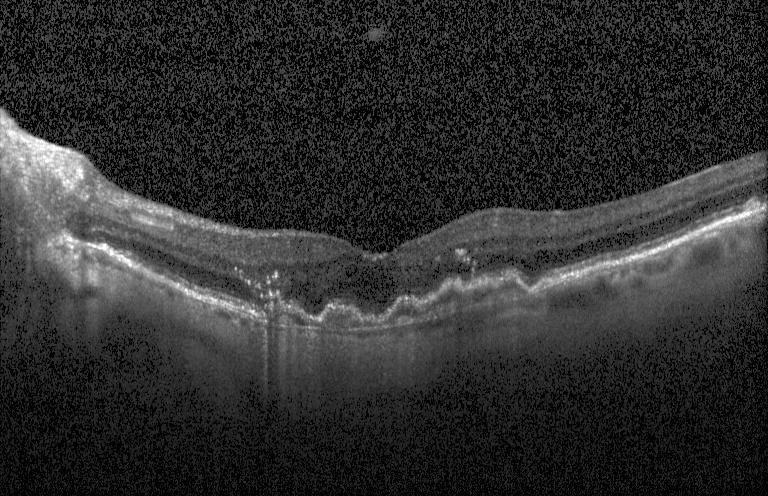 OCT B-scan showing choroidal neovascularization.